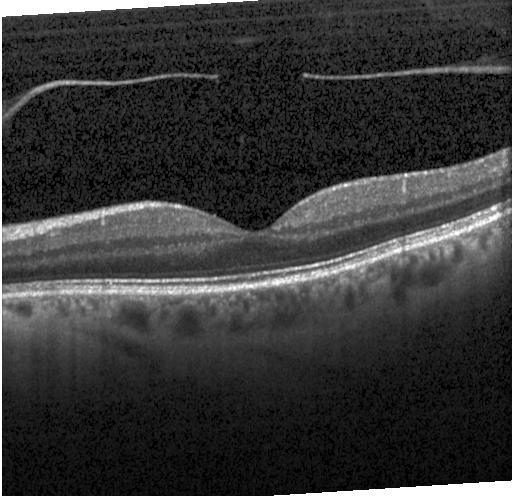
OCT B-scan showing no evidence of choroidal neovascularization, diabetic macular edema, or drusen.